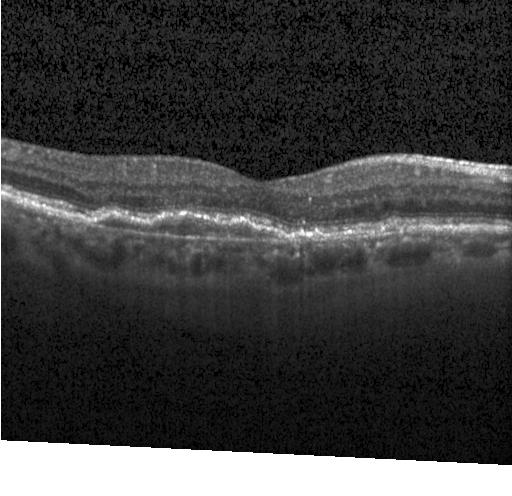
Heidelberg Spectralis OCT system, OCT line scan
Impression: choroidal neovascularization (CNV).